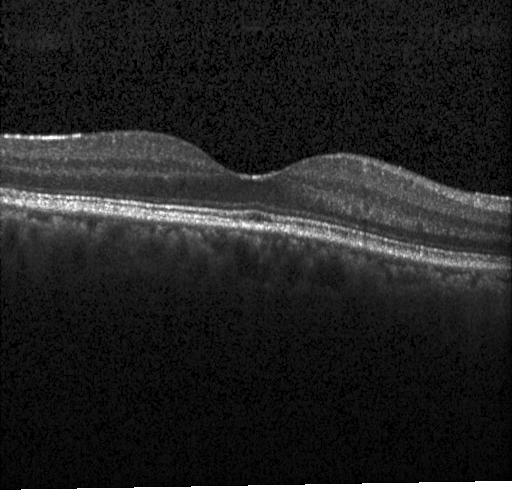 Retinal OCT B-scan.
Neither choroidal neovascularization, diabetic macular edema, nor drusen.